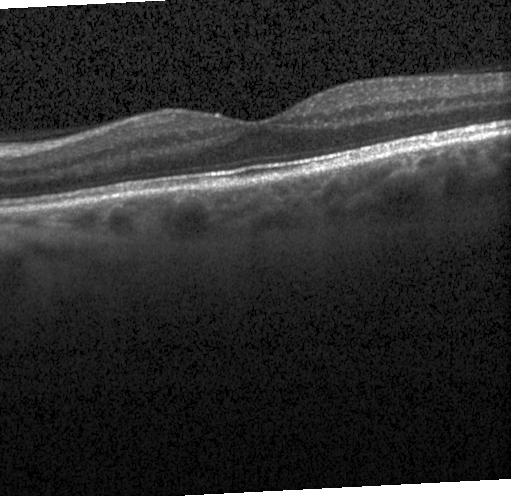 Centered on the fovea. OCT line scan. SD-OCT. The scan shows no evidence of CNV, DME, or drusen.